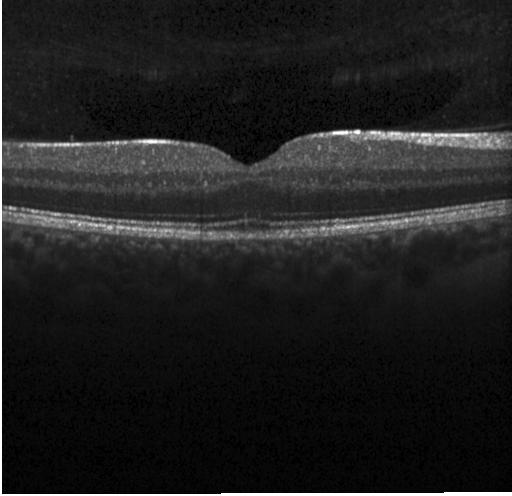

Retinal OCT cross-section; horizontal scan through the fovea; SD-OCT — This B-scan demonstrates no choroidal neovascularization, diabetic macular edema, or drusen.